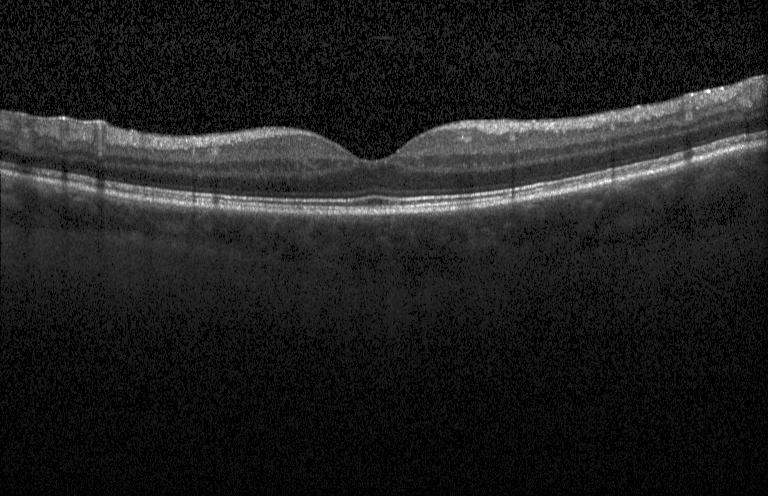

OCT B-scan.
Finding: neither choroidal neovascularization, diabetic macular edema, nor drusen.